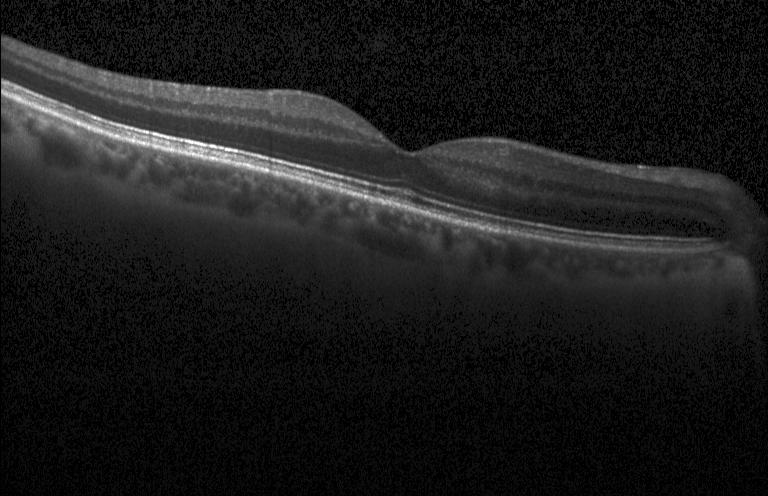
Heidelberg Spectralis, horizontal scan through the fovea, retinal OCT cross-section, spectral-domain optical coherence tomography.
OCT finding: neither choroidal neovascularization, diabetic macular edema, nor drusen.